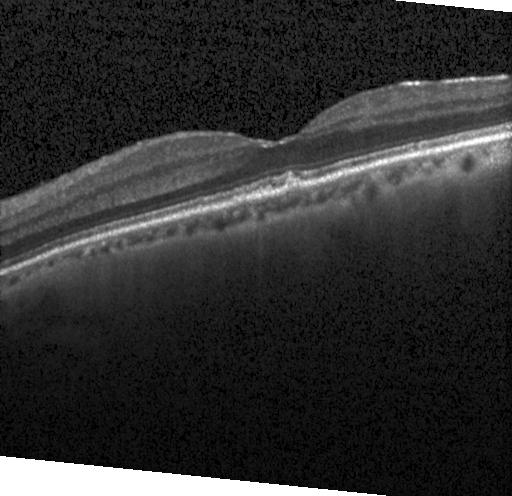

Macular scan, retinal OCT cross-section, acquired on a Heidelberg Spectralis — OCT finding: drusen.